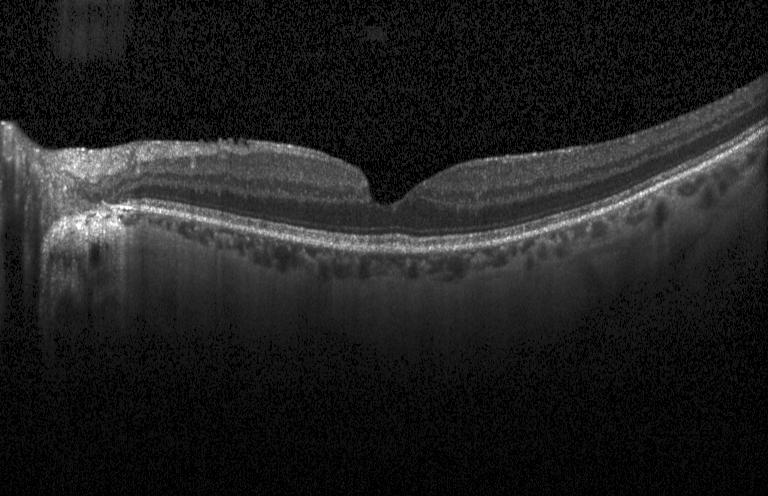
Diagnosis: no evidence of choroidal neovascularization, diabetic macular edema, or drusen.